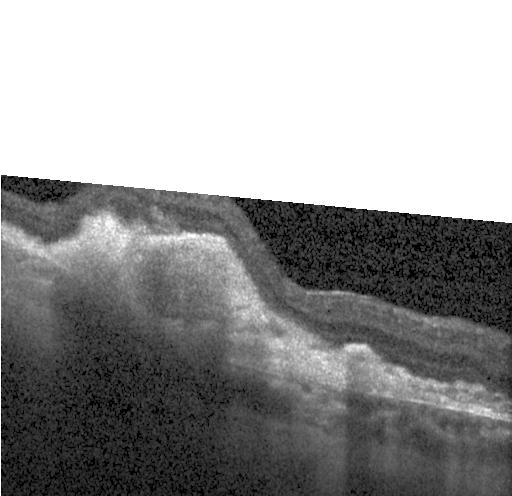
Retinal OCT cross-section; spectral-domain OCT — Diagnosis: choroidal neovascularization (CNV).